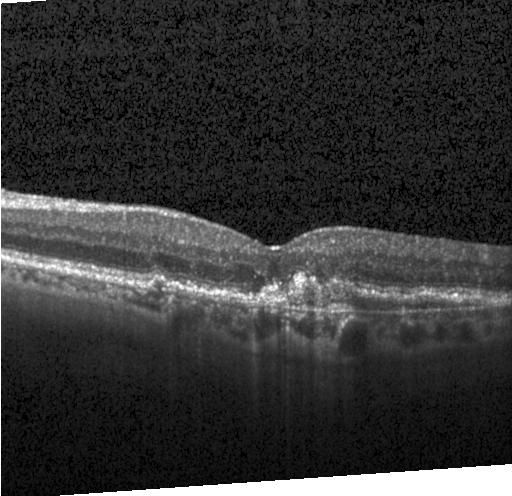 Diagnosis: a choroidal neovascular membrane.